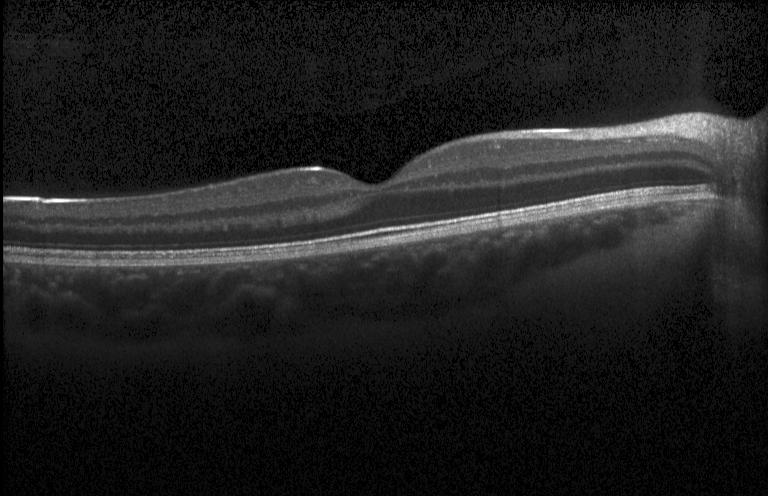

OCT finding: neither CNV, DME, nor drusen.